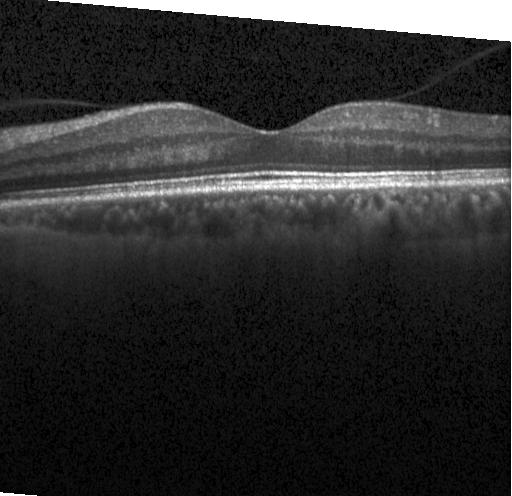
Spectral-domain OCT B-scan: neither choroidal neovascularization, diabetic macular edema, nor drusen.